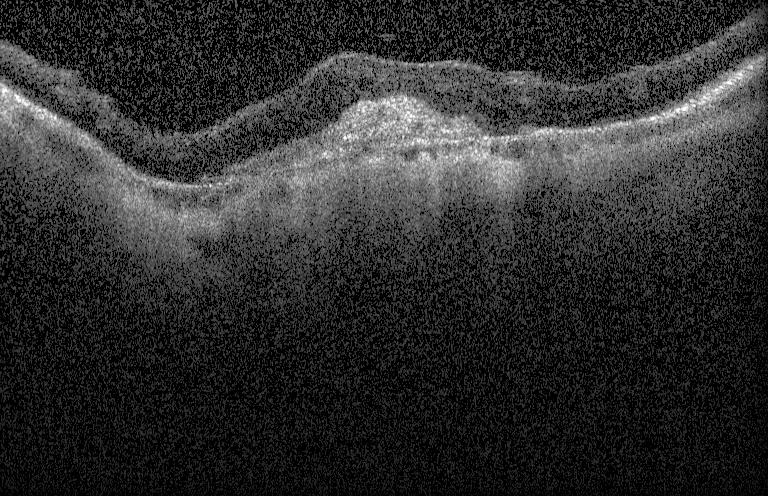 Diagnosis: CNV.